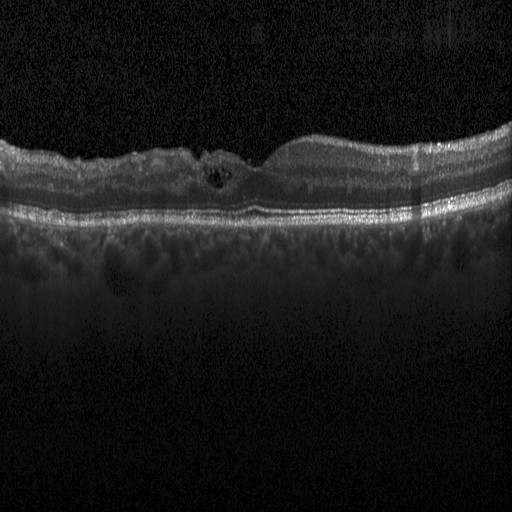
OCT B-scan — Finding: diabetic macular edema.